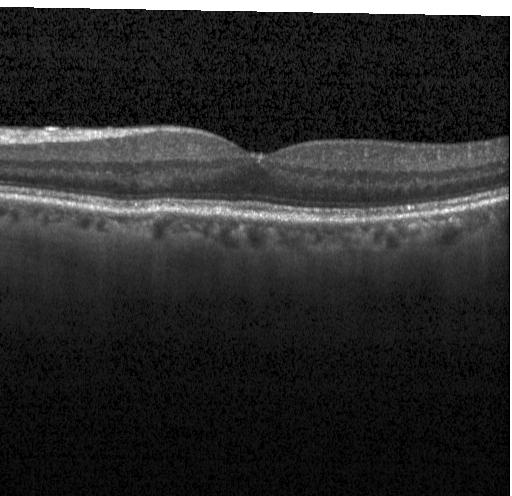

Assessment: neither CNV, DME, nor drusen.